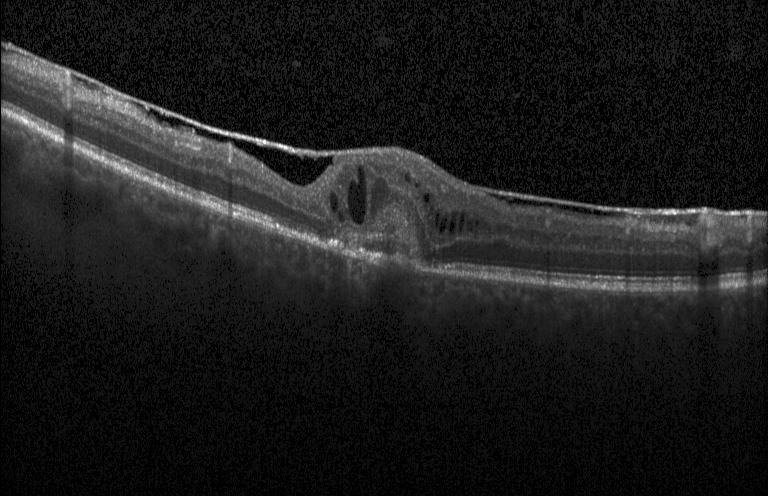

A choroidal neovascular membrane.